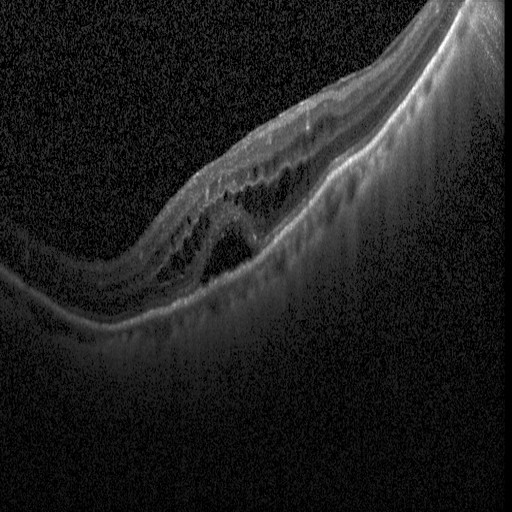
Optical coherence tomography B-scan.
Finding: diabetic macular edema.